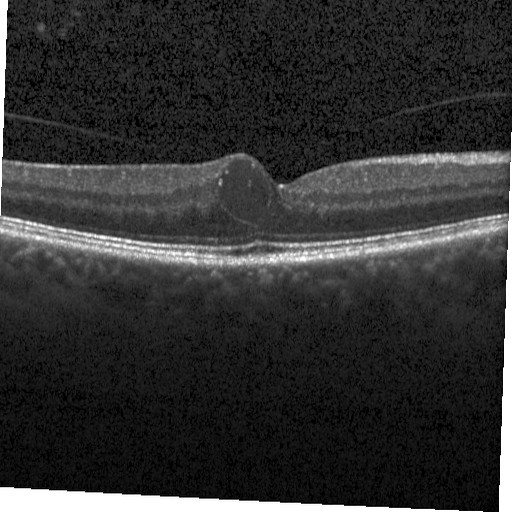 OCT B-scan.
Finding: diabetic macular edema (DME).